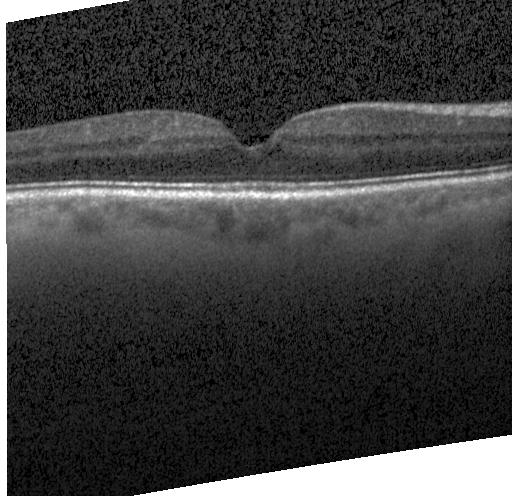 Retinal OCT cross-section.
OCT finding: neither choroidal neovascularization, diabetic macular edema, nor drusen.